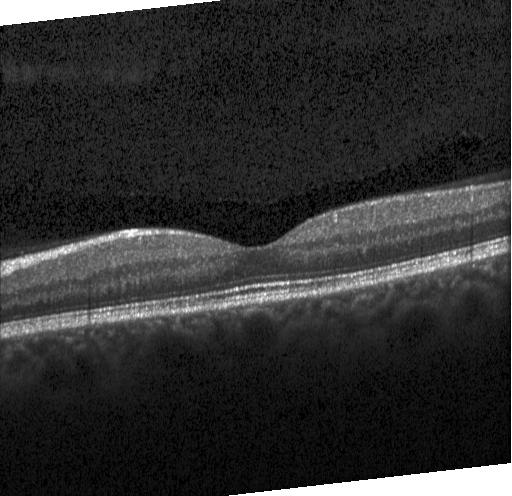
OCT scan showing no choroidal neovascularization, diabetic macular edema, or drusen.